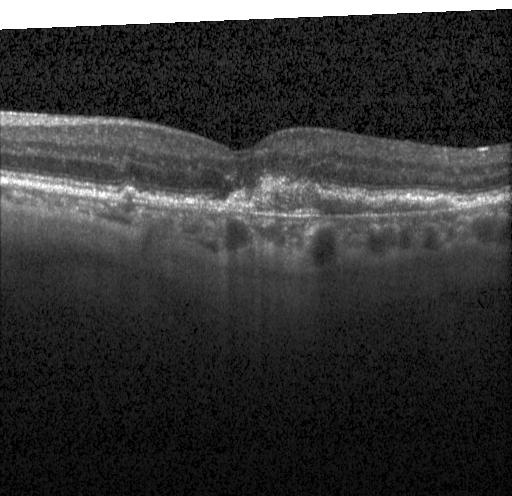 Retinal OCT B-scan.
Impression: choroidal neovascularization.